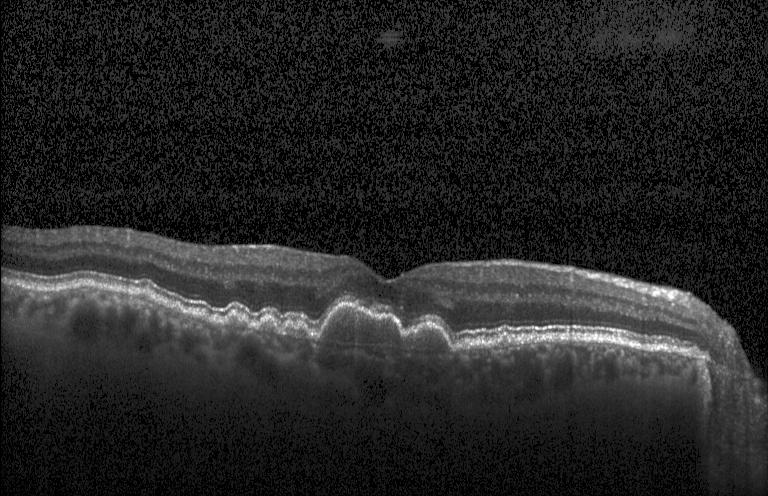 Macular OCT: multiple drusen.